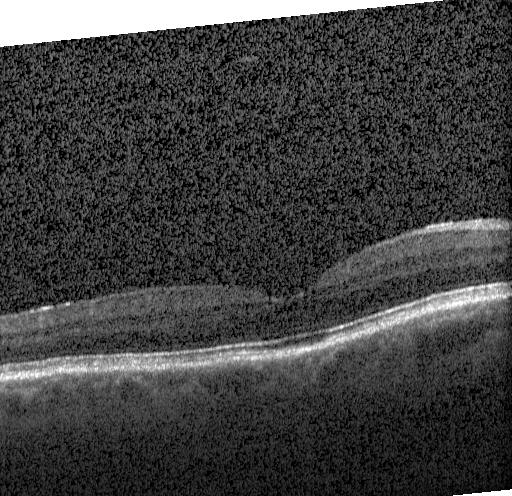 No choroidal neovascularization, diabetic macular edema, or drusen.